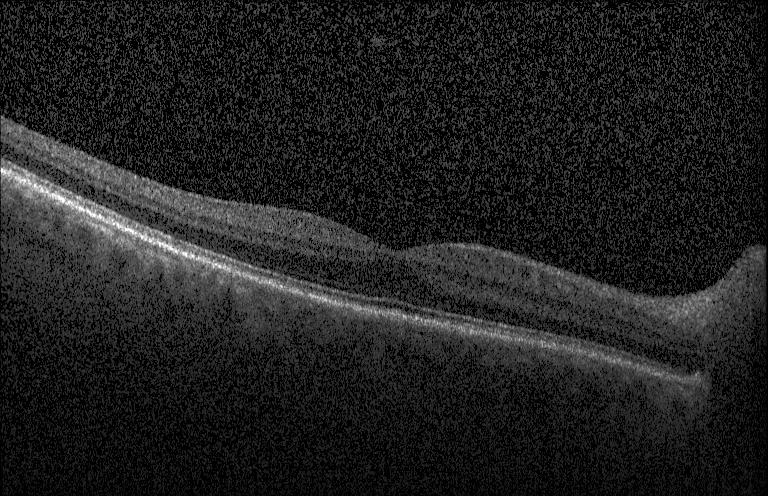

Dx: no CNV, DME, or drusen.